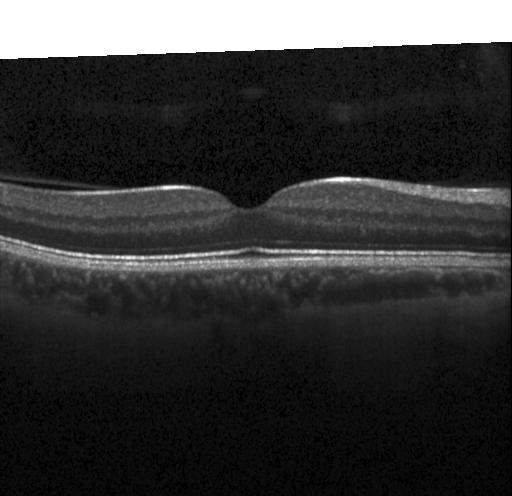

Optical coherence tomography B-scan · spectral-domain OCT. No choroidal neovascularization, no diabetic macular edema, and no drusen.